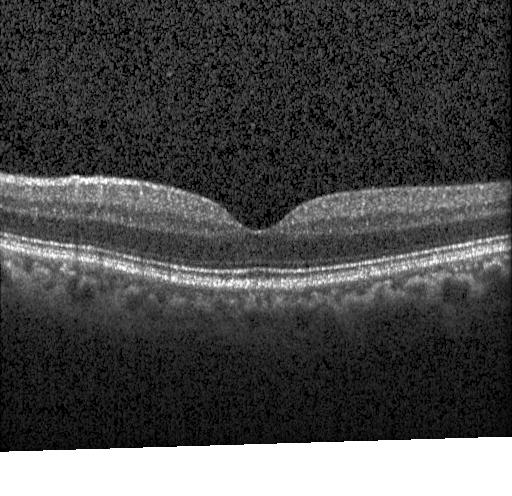
Optical coherence tomography B-scan, fovea-centered
Assessment: no evidence of choroidal neovascularization, diabetic macular edema, or drusen.